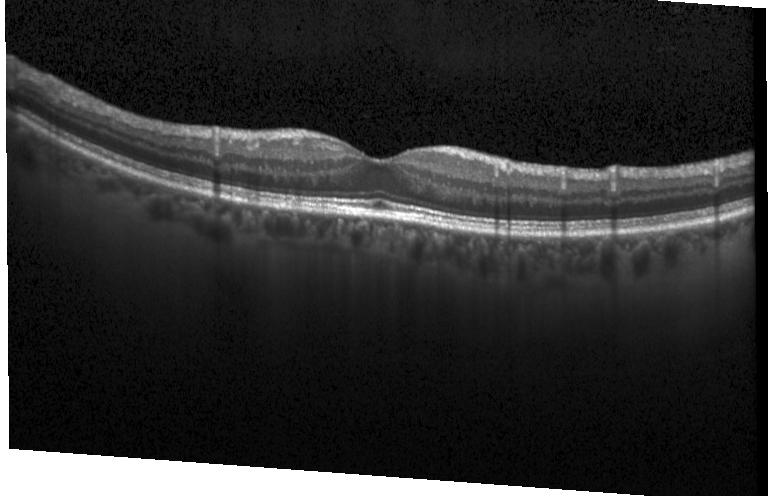 Optical coherence tomography scan
Finding: no evidence of choroidal neovascularization, diabetic macular edema, or drusen.